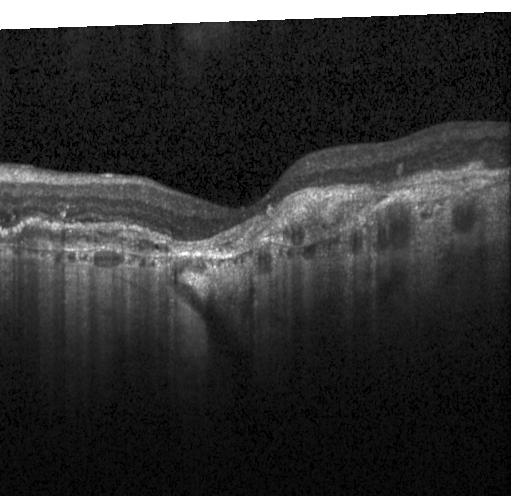
Optical coherence tomography B-scan, SD-OCT.
Impression: a choroidal neovascular membrane.